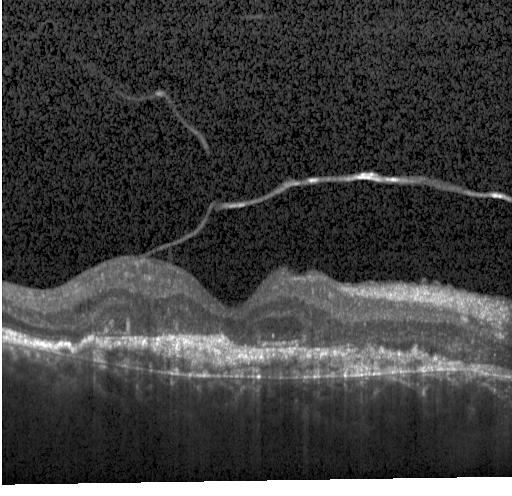 Through the macula; optical coherence tomography B-scan; spectral-domain OCT; acquired on a Heidelberg Spectralis
The scan shows choroidal neovascularization (CNV).